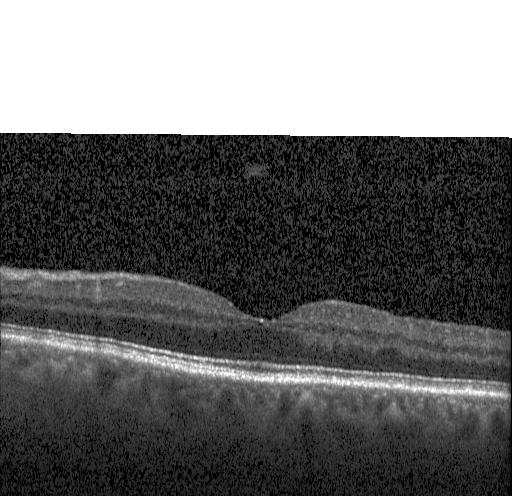
Impression: no choroidal neovascularization, no diabetic macular edema, and no drusen.